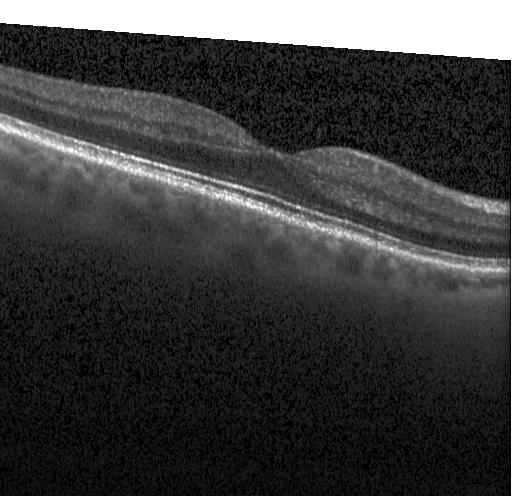

Optical coherence tomography scan, macular scan, spectral-domain optical coherence tomography.
Finding: no CNV, no DME, and no drusen.